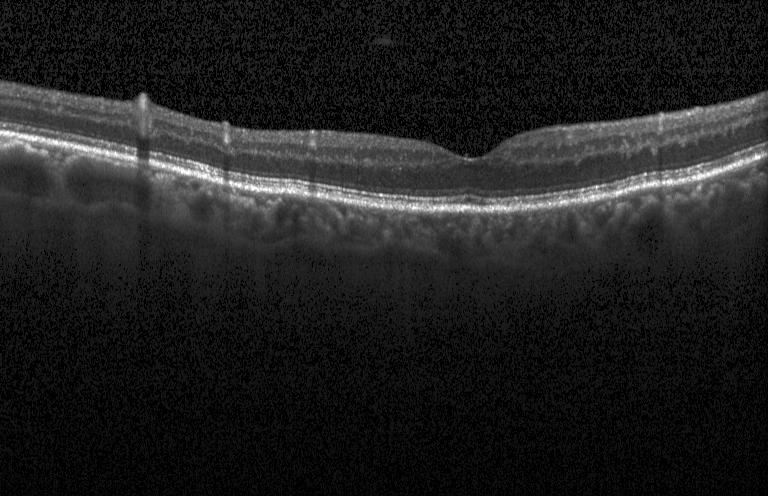 Assessment: no CNV, DME, or drusen.